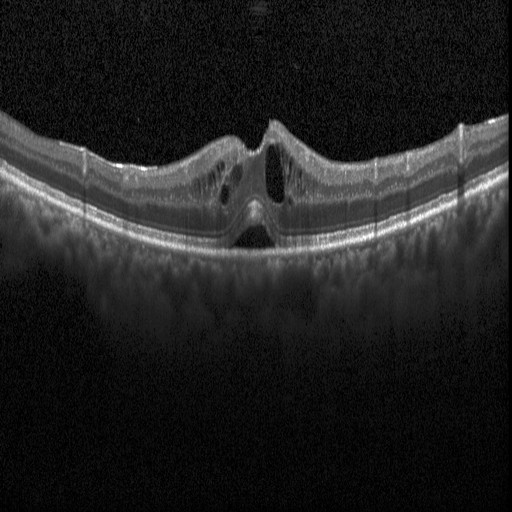

OCT finding: DME.